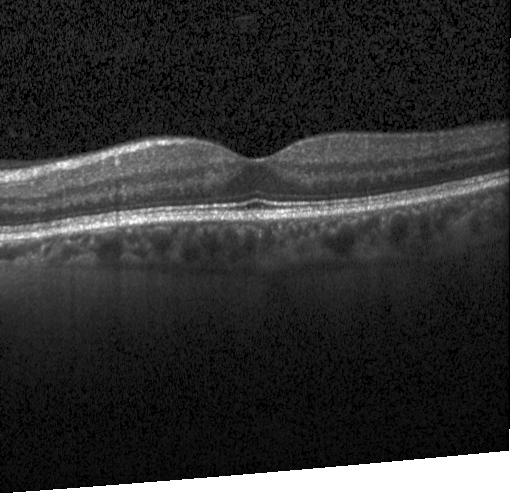
Macular OCT: no evidence of choroidal neovascularization, diabetic macular edema, or drusen.